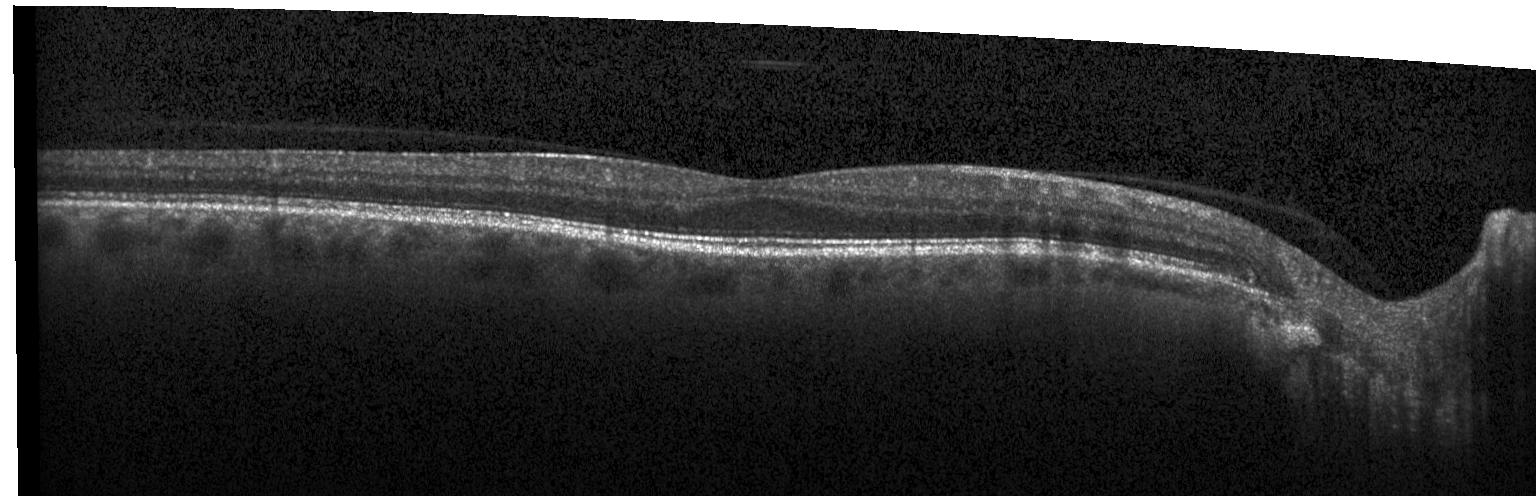

Instrument: Heidelberg Spectralis. OCT B-scan
Impression: no evidence of choroidal neovascularization, diabetic macular edema, or drusen.